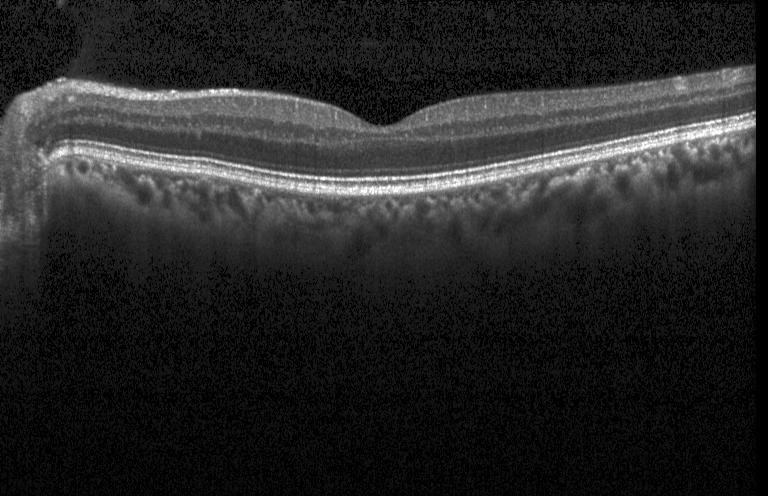
This B-scan demonstrates neither CNV, DME, nor drusen.